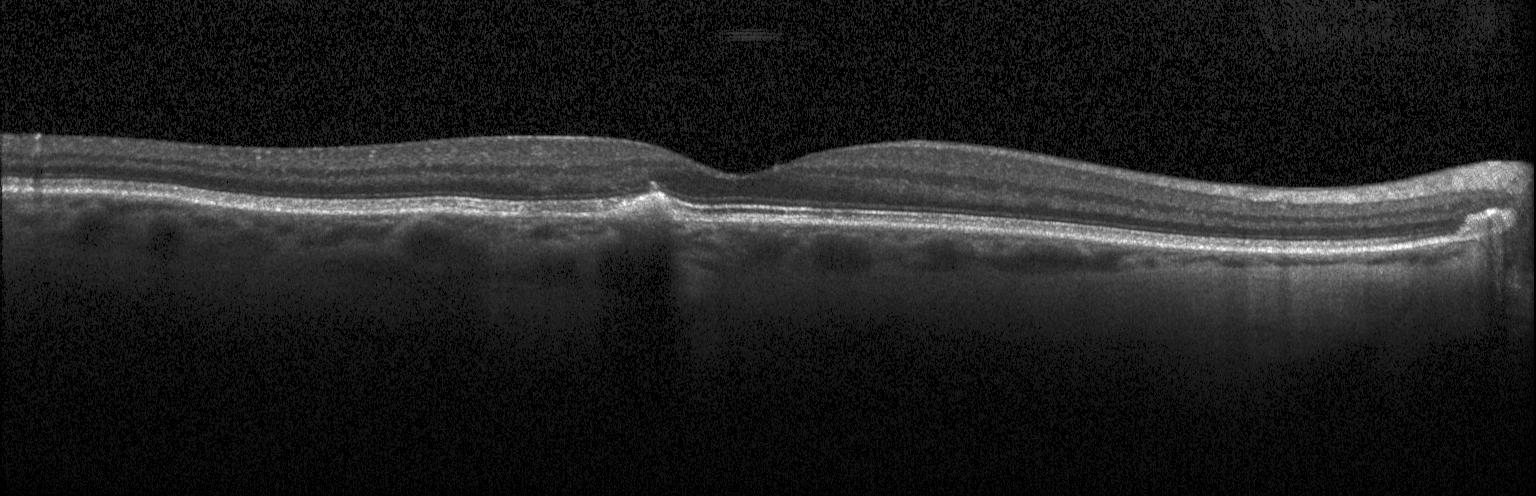 Dx: drusen.